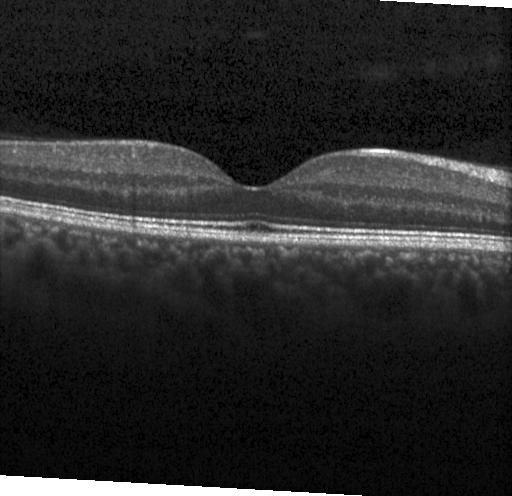
Through the macula. Retinal OCT cross-section. Spectral-domain OCT — Finding: neither CNV, DME, nor drusen.